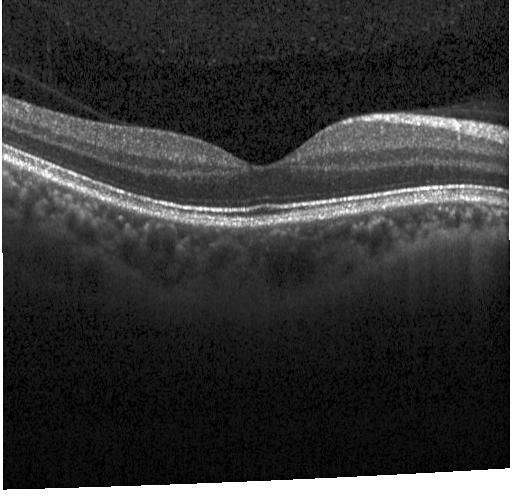

SD-OCT. Optical coherence tomography scan. Heidelberg Spectralis OCT system. Macular scan.
Finding: no choroidal neovascularization, no diabetic macular edema, and no drusen.